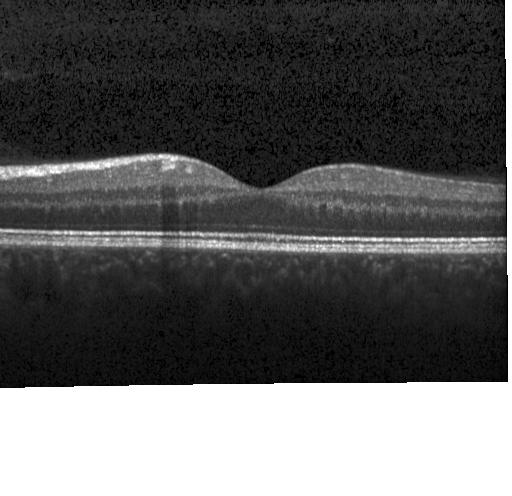
OCT B-scan, instrument: Heidelberg Spectralis, horizontal scan through the fovea
Diagnosis: no CNV, DME, or drusen.